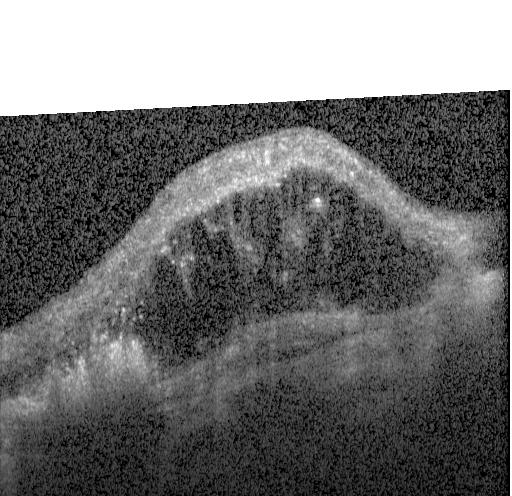

Dx: diabetic macular edema.